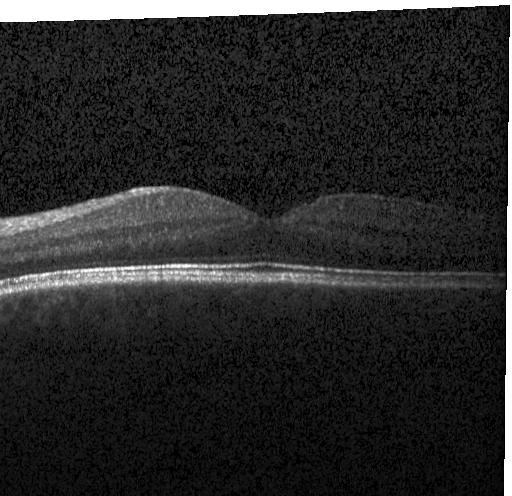
Impression: neither choroidal neovascularization, diabetic macular edema, nor drusen.